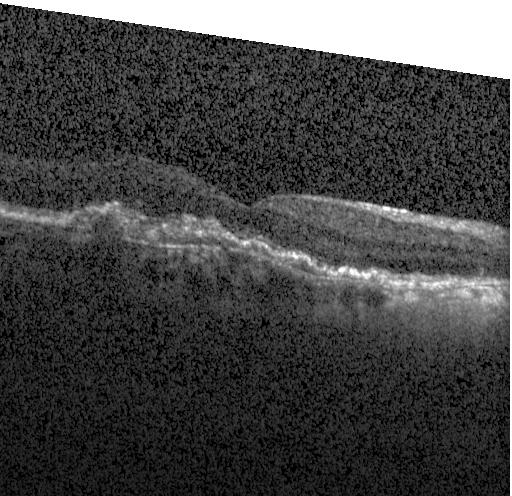

SD-OCT. Fovea-centered. OCT B-scan. Instrument: Heidelberg Spectralis
Diagnosis: CNV.